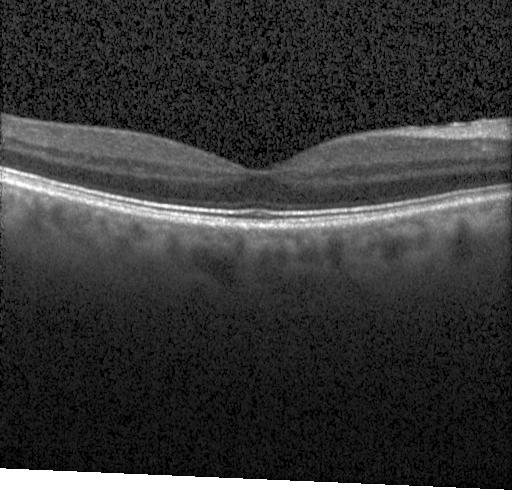 Fovea-centered. Optical coherence tomography scan. Impression: neither choroidal neovascularization, diabetic macular edema, nor drusen.